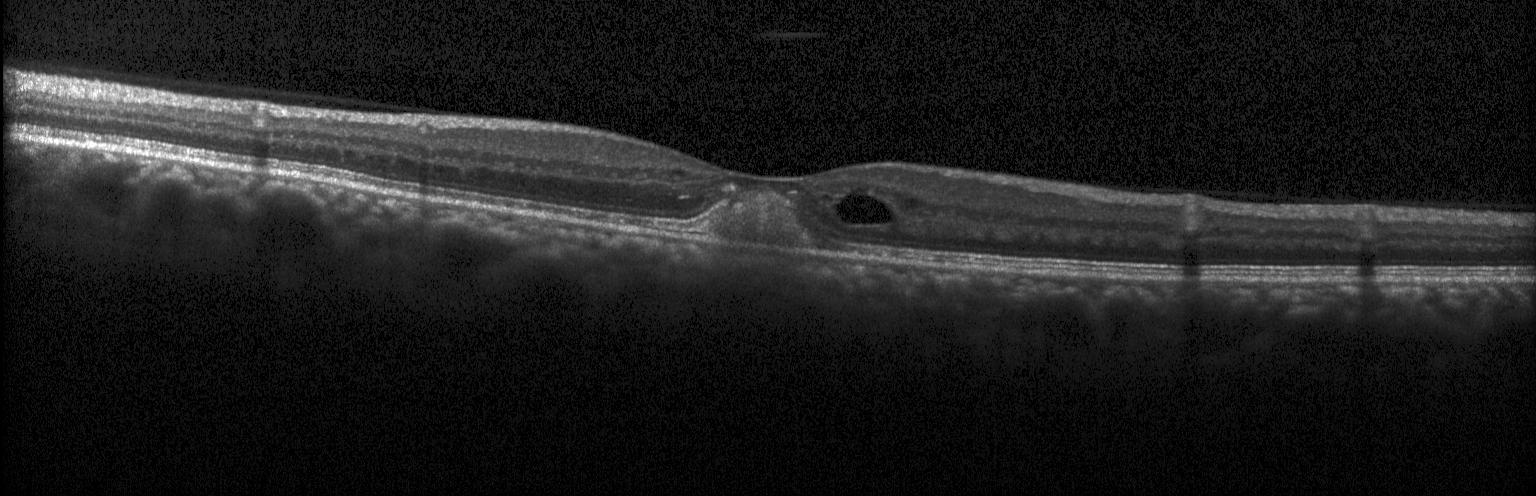 Optical coherence tomography scan — Diagnosis: choroidal neovascularization (CNV).